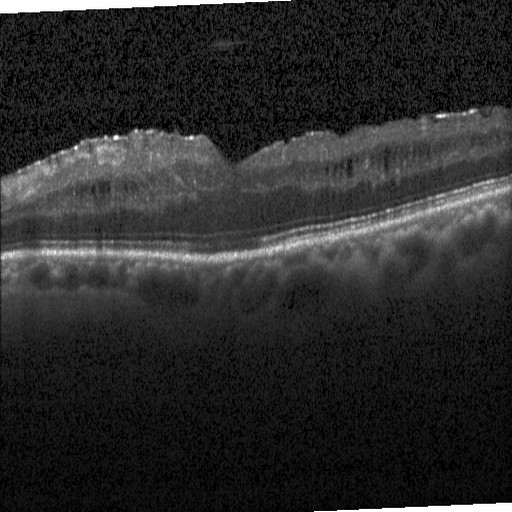 Assessment: diabetic macular edema (DME).